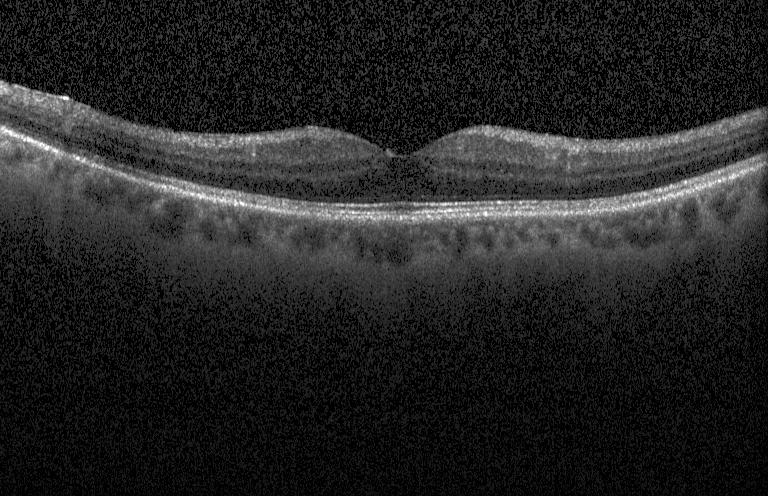

Retinal OCT B-scan, Heidelberg Spectralis OCT system, spectral-domain OCT, macular scan. Finding: no CNV, no DME, and no drusen.